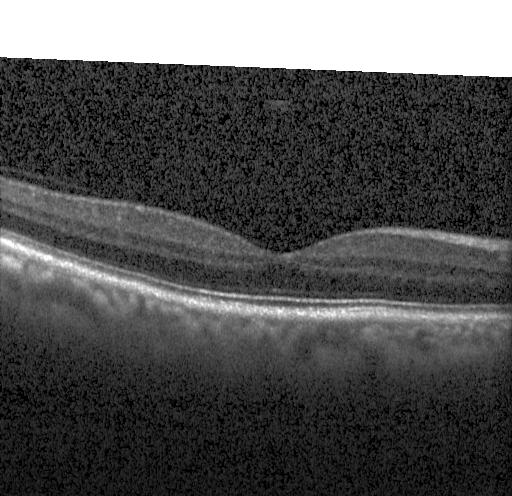

Impression: neither choroidal neovascularization, diabetic macular edema, nor drusen.